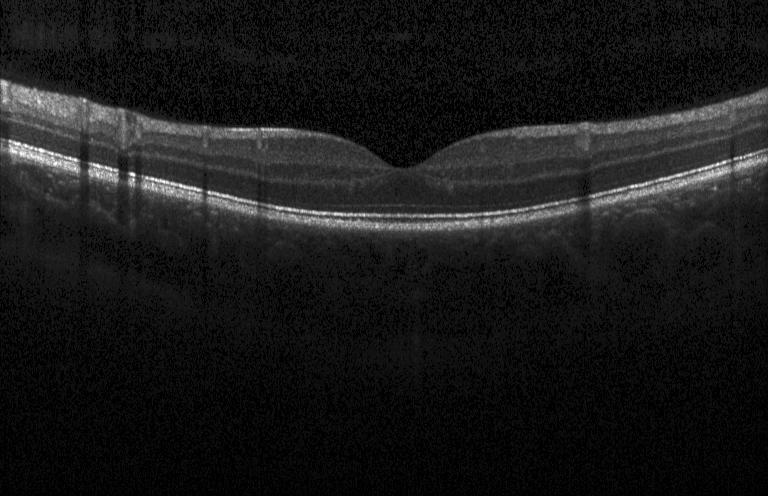 No evidence of choroidal neovascularization, diabetic macular edema, or drusen.